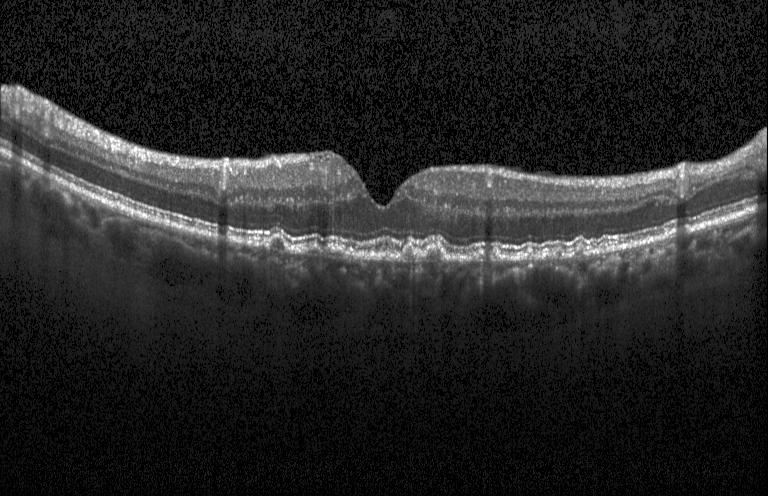

This B-scan demonstrates multiple drusen.